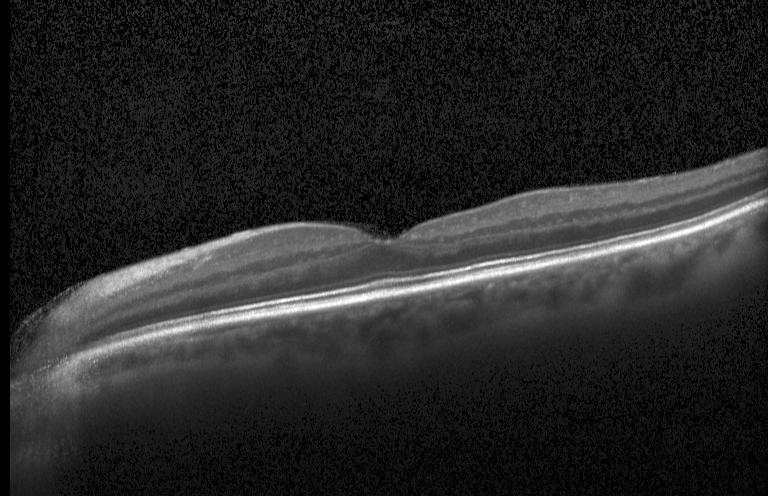

Diagnosis: neither choroidal neovascularization, diabetic macular edema, nor drusen.